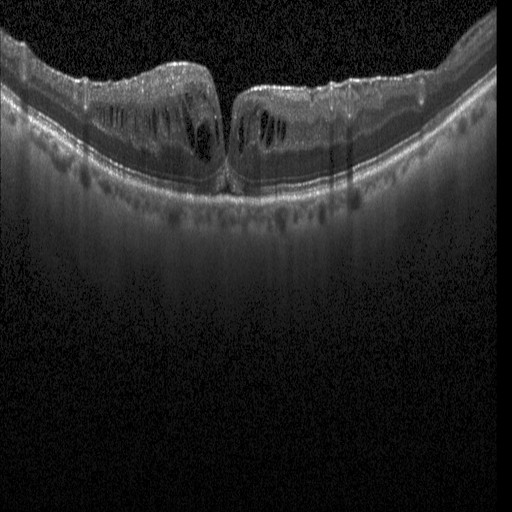

Retinal OCT B-scan, fovea-centered
OCT finding: diabetic macular edema.